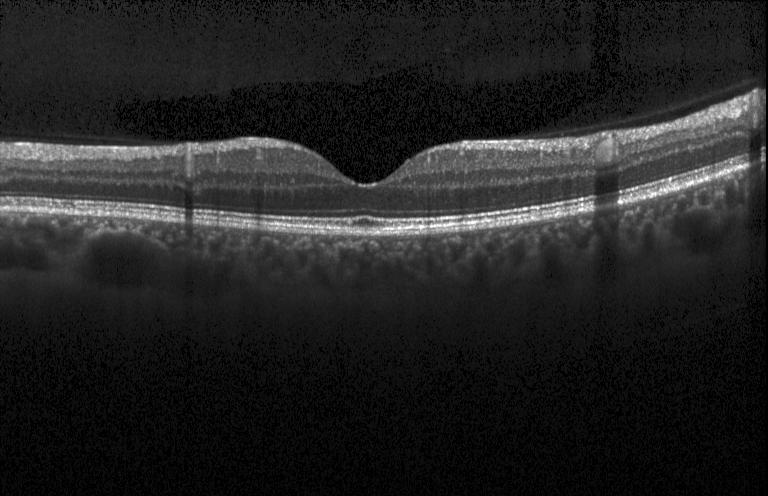

Macular OCT: no evidence of choroidal neovascularization, diabetic macular edema, or drusen.